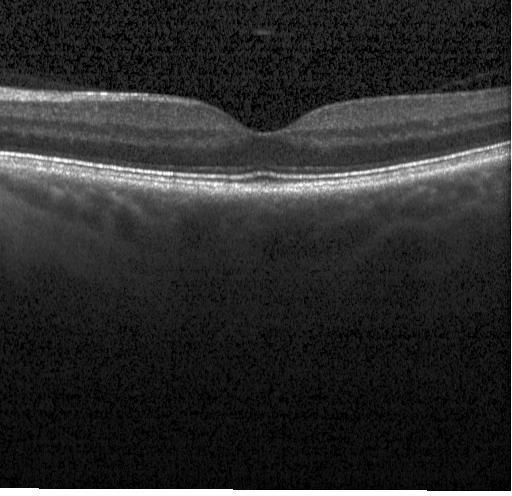

Instrument: Heidelberg Spectralis. Spectral-domain OCT. Optical coherence tomography scan. Horizontal scan through the fovea.
Assessment: no evidence of choroidal neovascularization, diabetic macular edema, or drusen.